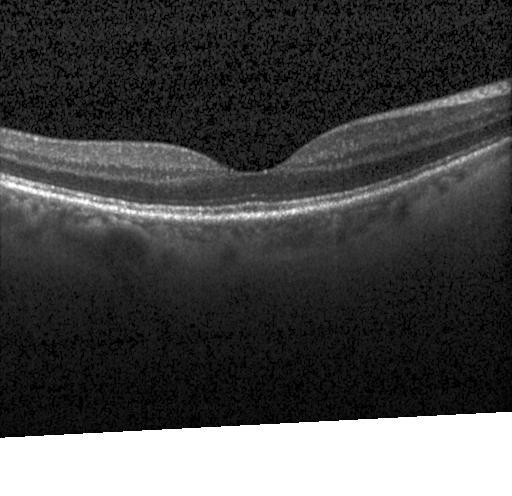
Spectral-domain optical coherence tomography · retinal OCT B-scan · instrument: Heidelberg Spectralis
No CNV, no DME, and no drusen.